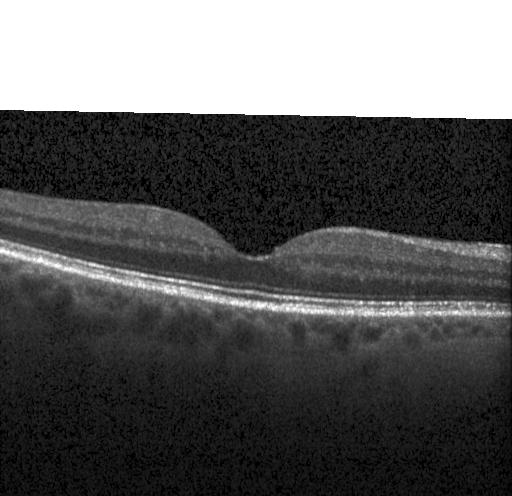 Spectral-domain OCT B-scan: no choroidal neovascularization, no diabetic macular edema, and no drusen.